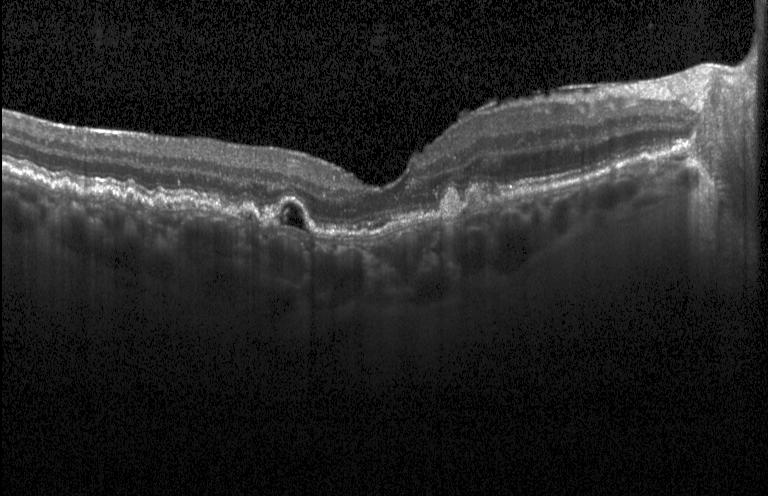
Spectral-domain OCT B-scan: a choroidal neovascular membrane.